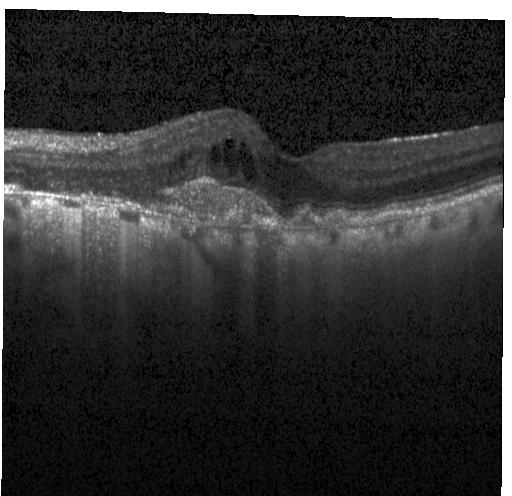

Horizontal scan through the fovea · spectral-domain OCT · optical coherence tomography B-scan · acquired on a Heidelberg Spectralis.
Dx: choroidal neovascularization.